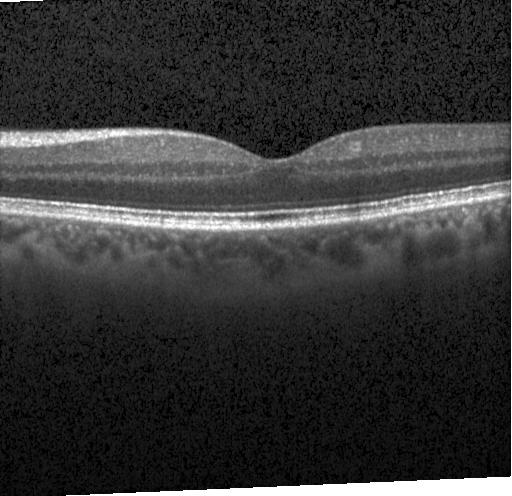

Retinal OCT B-scan · instrument: Heidelberg Spectralis
OCT finding: neither choroidal neovascularization, diabetic macular edema, nor drusen.